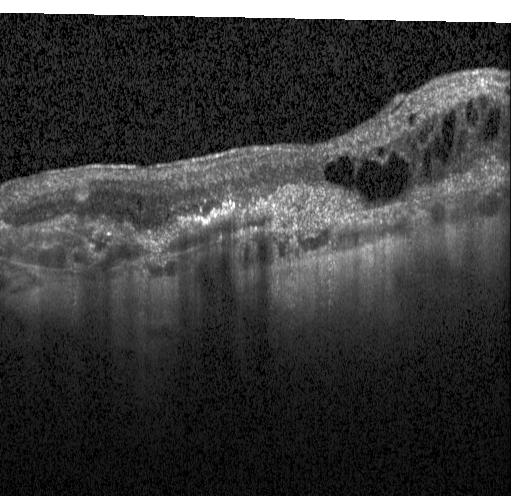 CNV.